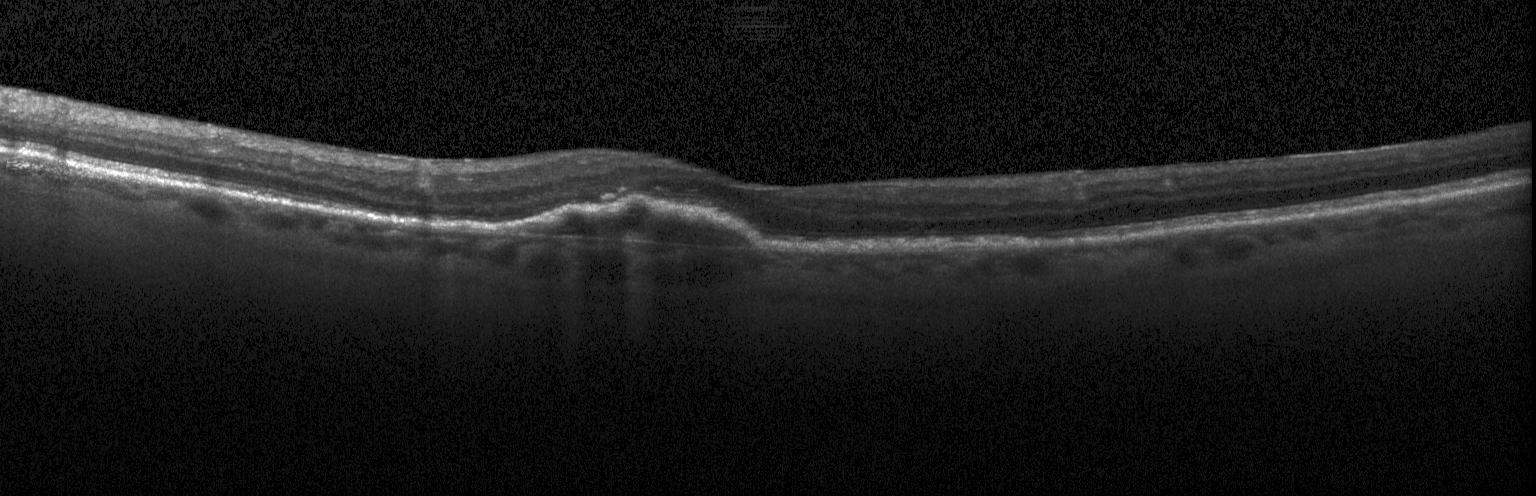

Finding: choroidal neovascularization (CNV).